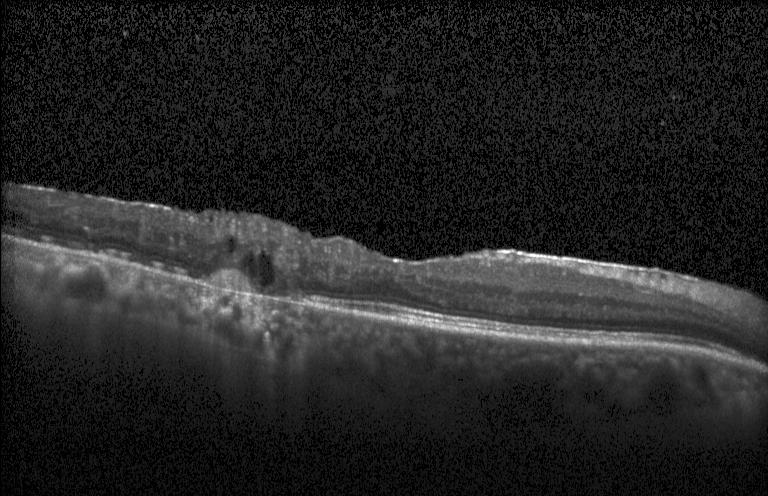 OCT line scan; spectral-domain optical coherence tomography — Finding: a choroidal neovascular membrane.